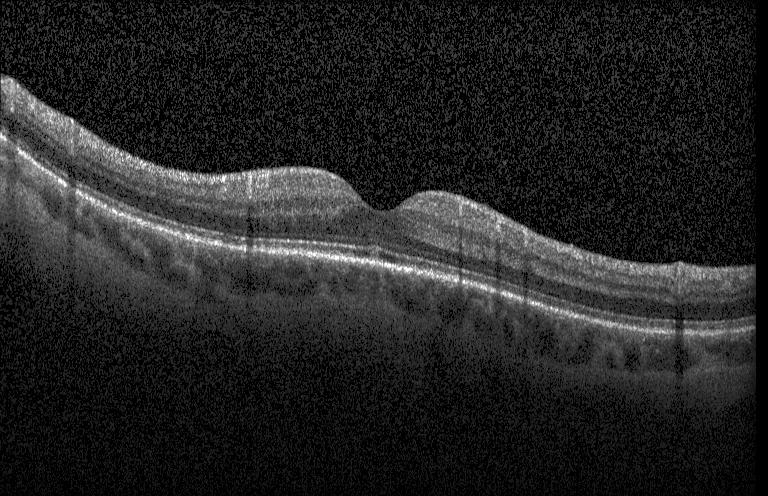 Finding: no evidence of choroidal neovascularization, diabetic macular edema, or drusen.